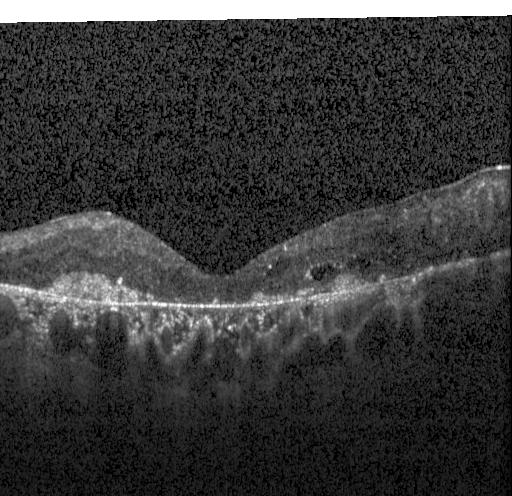 Through the macula, retinal OCT cross-section. This B-scan demonstrates choroidal neovascularization.